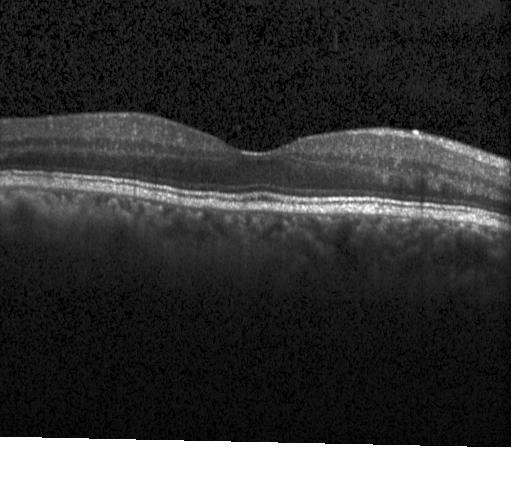
Heidelberg Spectralis · retinal OCT B-scan.
Finding: no CNV, DME, or drusen.